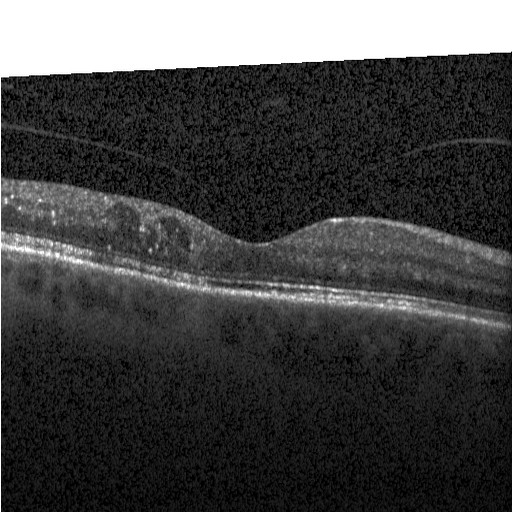

Retinal OCT B-scan — Macular OCT: DME.